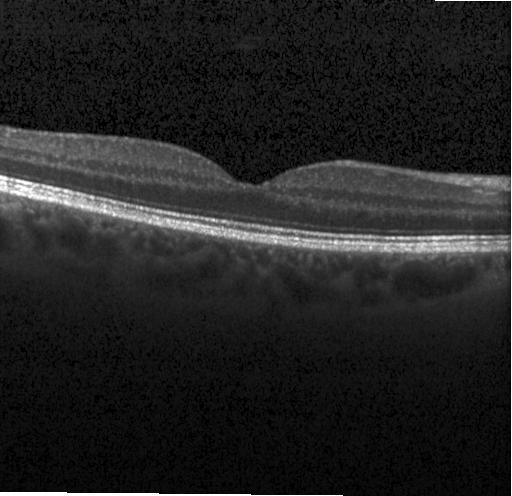
Optical coherence tomography scan.
Diagnosis: neither choroidal neovascularization, diabetic macular edema, nor drusen.